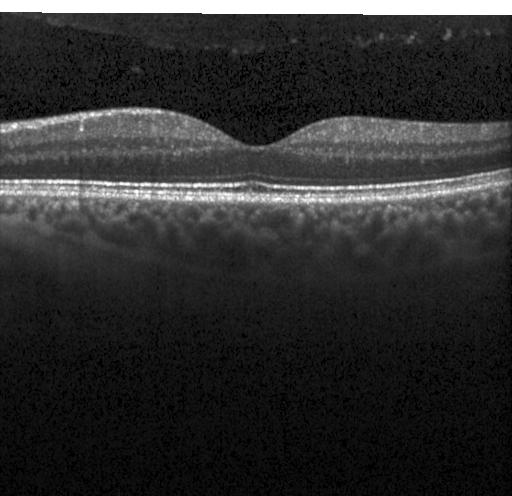
Macular OCT: no evidence of choroidal neovascularization, diabetic macular edema, or drusen.